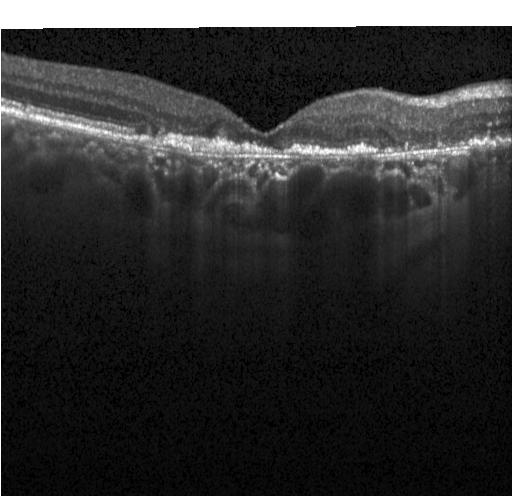
Retinal OCT cross-section. Instrument: Heidelberg Spectralis. Horizontal scan through the fovea. Dx: a choroidal neovascular membrane.